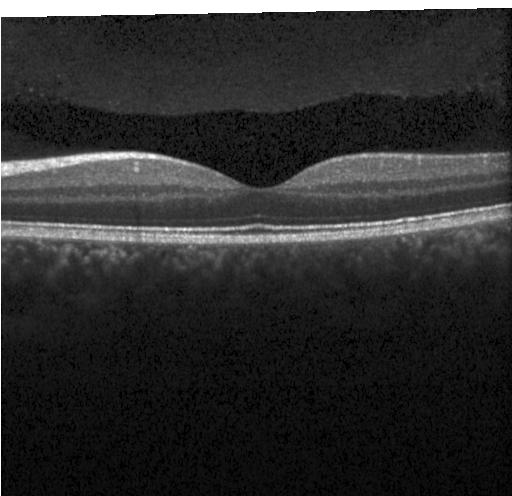

Retinal OCT B-scan — The scan shows neither choroidal neovascularization, diabetic macular edema, nor drusen.